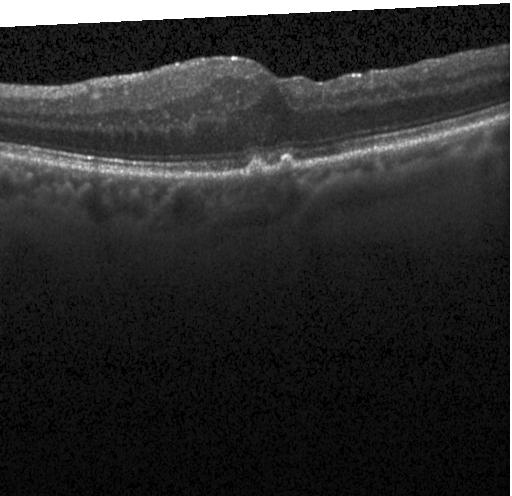

Fovea-centered; spectral-domain optical coherence tomography; instrument: Heidelberg Spectralis; retinal OCT cross-section.
Finding: drusen.